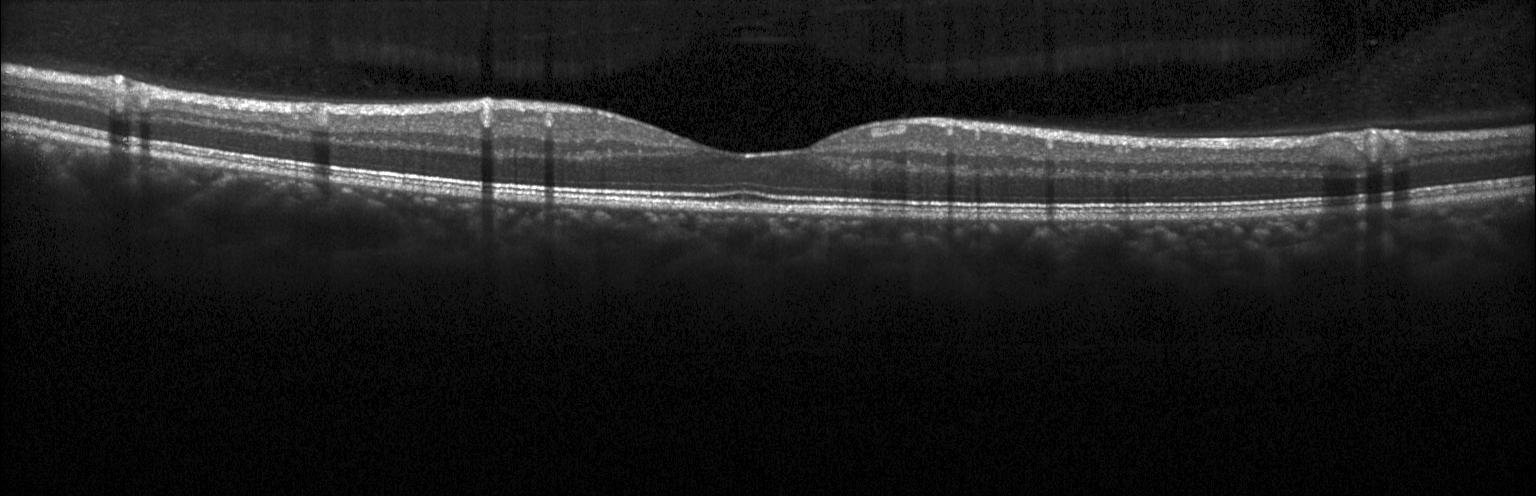
Finding: no evidence of choroidal neovascularization, diabetic macular edema, or drusen.